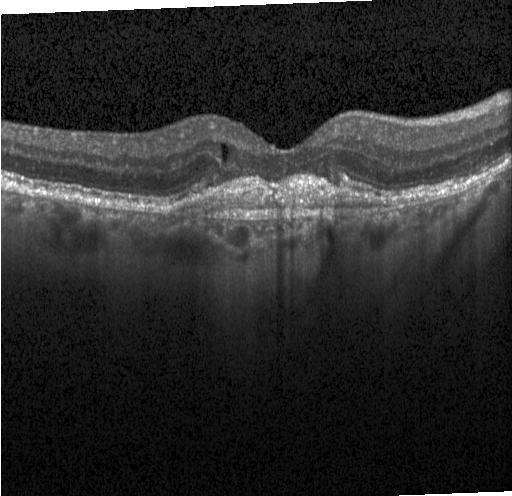

OCT B-scan showing a choroidal neovascular membrane.